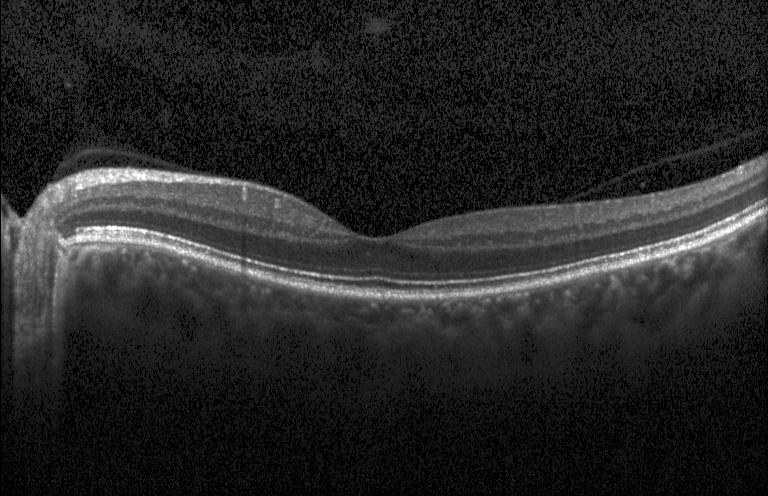 Retinal OCT B-scan, instrument: Heidelberg Spectralis — Neither CNV, DME, nor drusen.